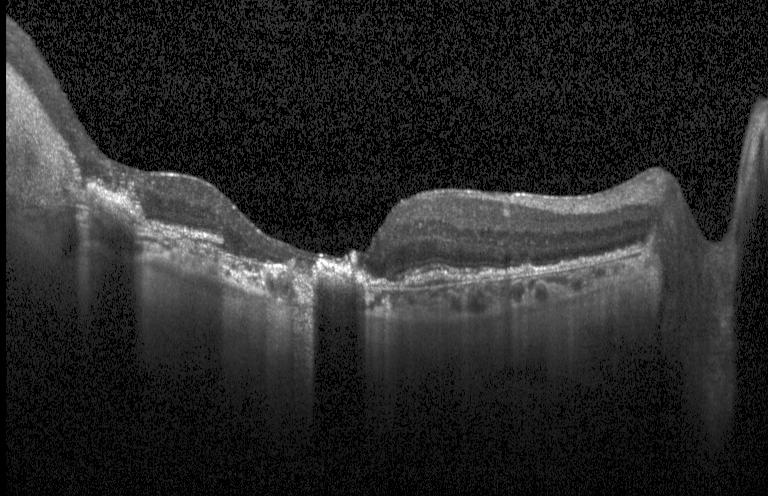

OCT finding: a choroidal neovascular membrane.